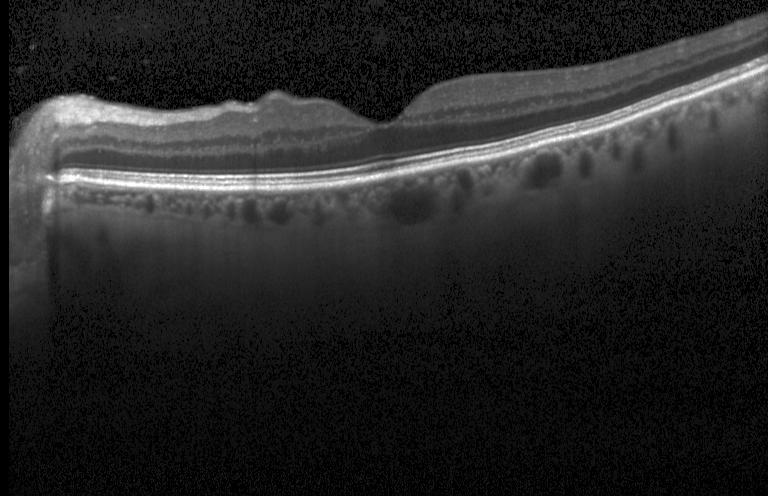 Retinal OCT cross-section. Macular scan. SD-OCT.
Impression: neither CNV, DME, nor drusen.